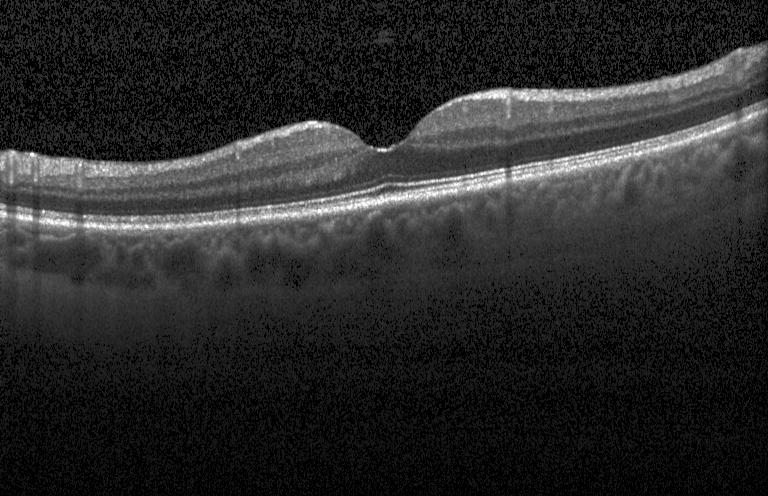
OCT scan showing no CNV, no DME, and no drusen.